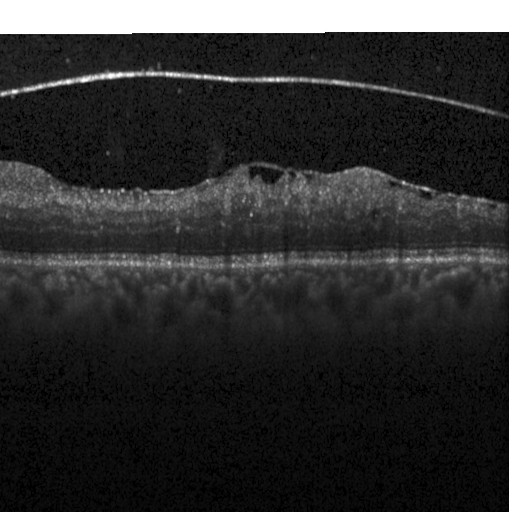
Impression: diabetic macular edema.